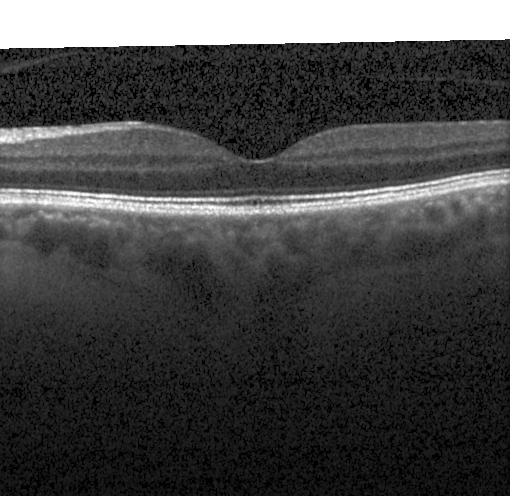 Spectral-domain OCT B-scan: no choroidal neovascularization, diabetic macular edema, or drusen.